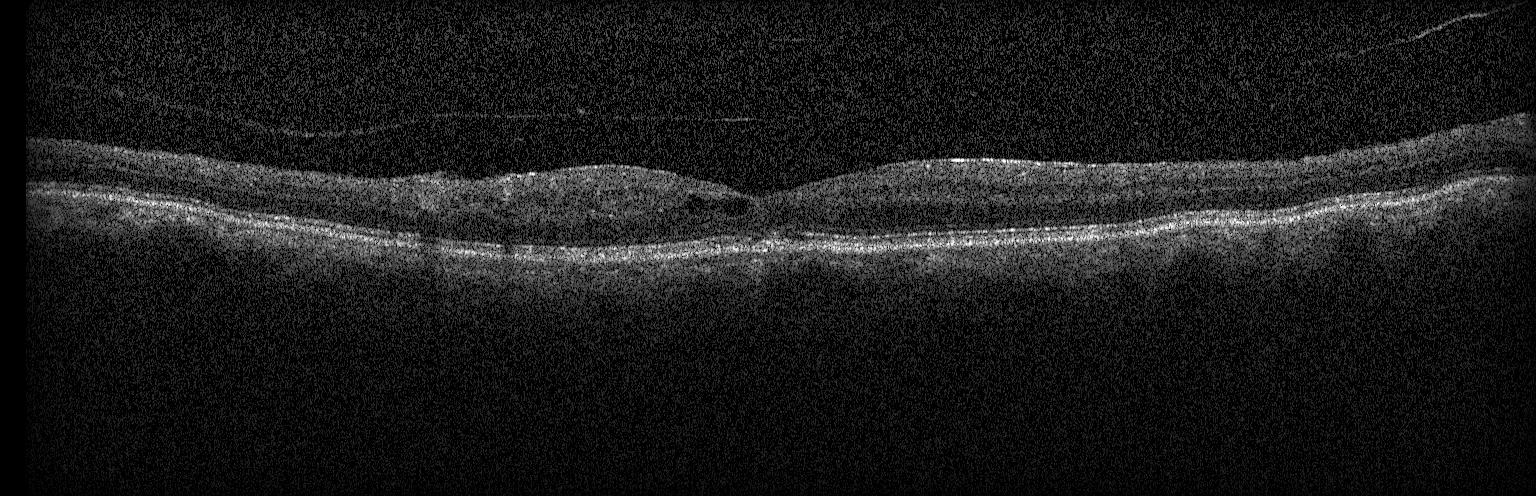

The scan shows diabetic macular edema.